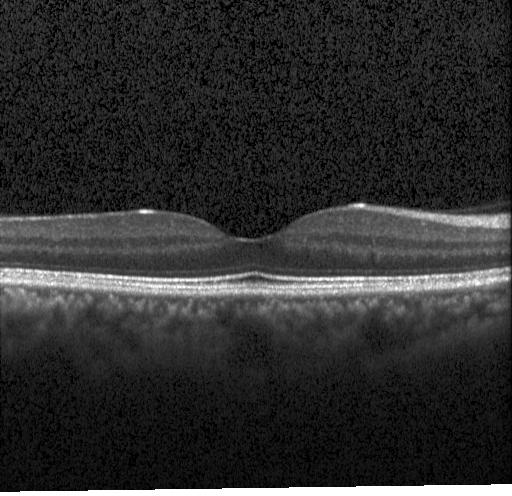

Diagnosis: neither CNV, DME, nor drusen.